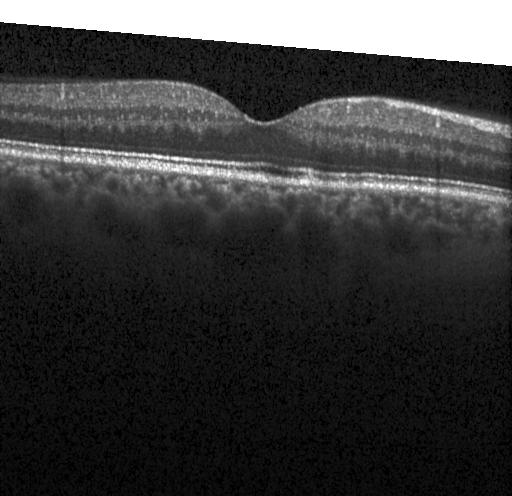
OCT line scan. Impression: no CNV, DME, or drusen.